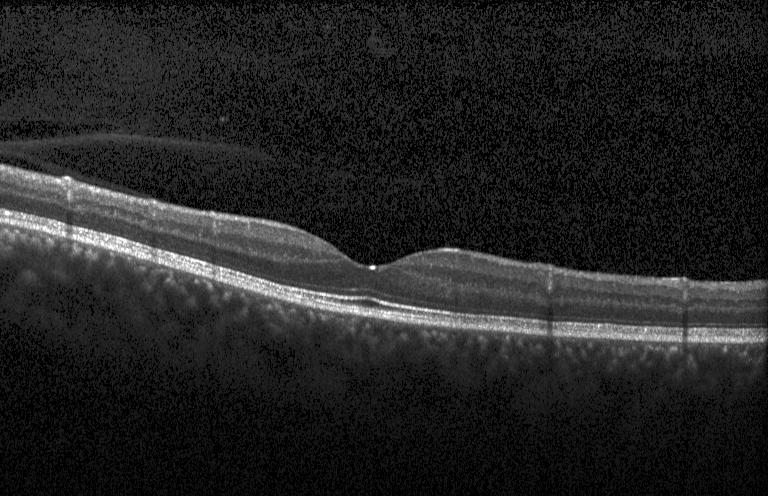
Retinal OCT B-scan · through the macula · Heidelberg Spectralis OCT system.
The scan shows no choroidal neovascularization, diabetic macular edema, or drusen.